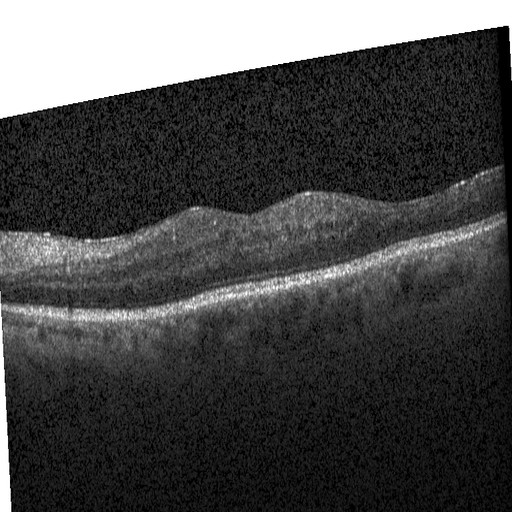 OCT B-scan; instrument: Heidelberg Spectralis. This B-scan demonstrates diabetic macular edema.